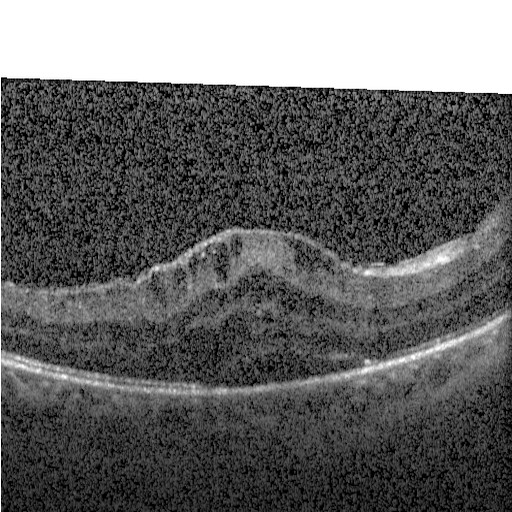
Assessment: diabetic macular edema.